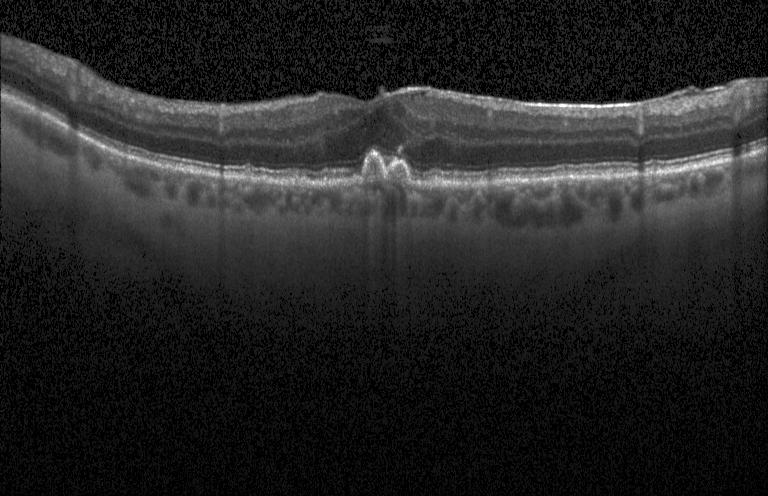

Dx: drusen.